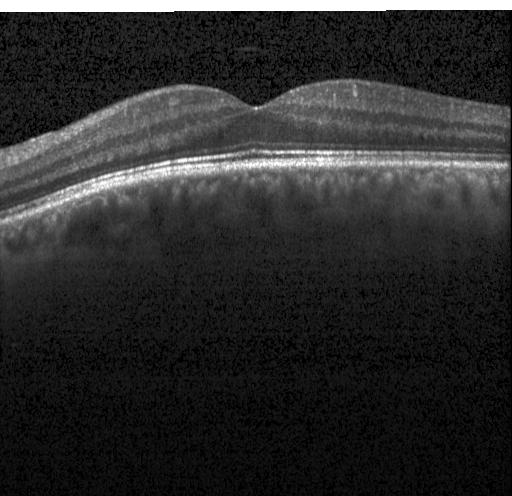

Diagnosis: no evidence of CNV, DME, or drusen.